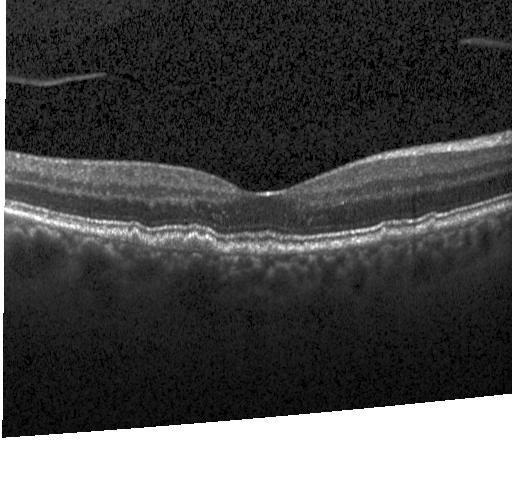 Optical coherence tomography scan — Impression: multiple drusen.